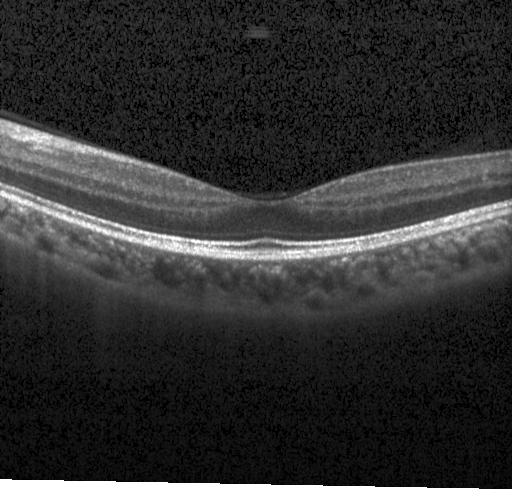

Retinal OCT cross-section showing no CNV, no DME, and no drusen.